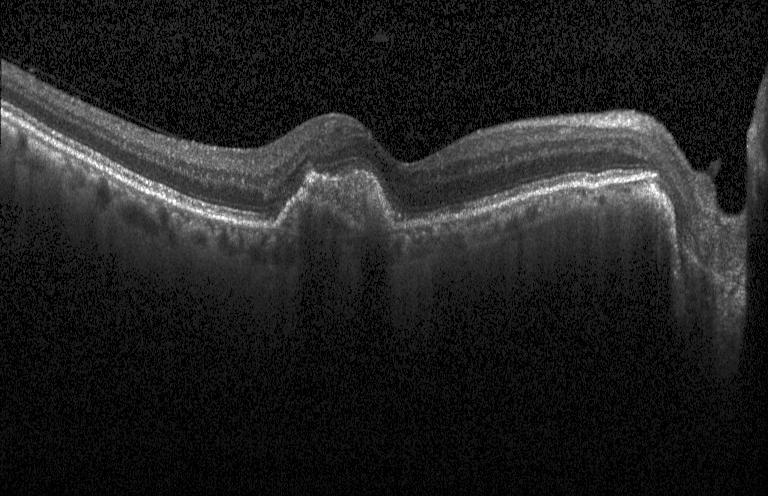
Retinal OCT B-scan. Assessment: a choroidal neovascular membrane.